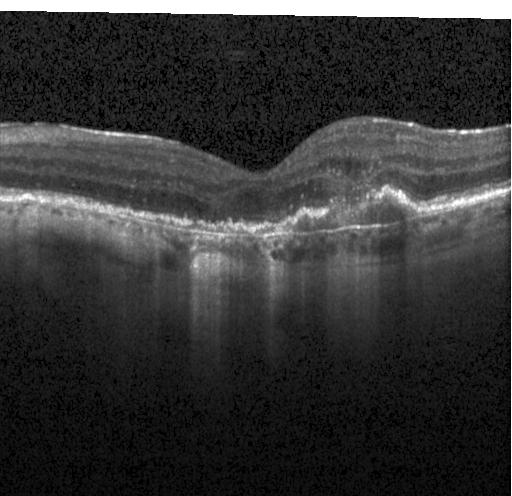
Diagnosis: a choroidal neovascular membrane.